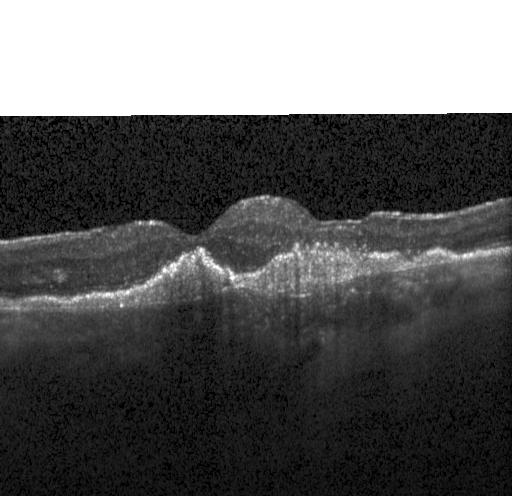

Macular OCT: CNV.